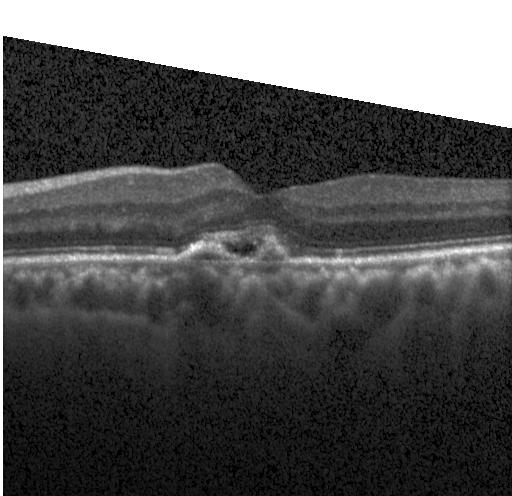 SD-OCT; centered on the fovea; retinal OCT cross-section — Assessment: choroidal neovascularization (CNV).